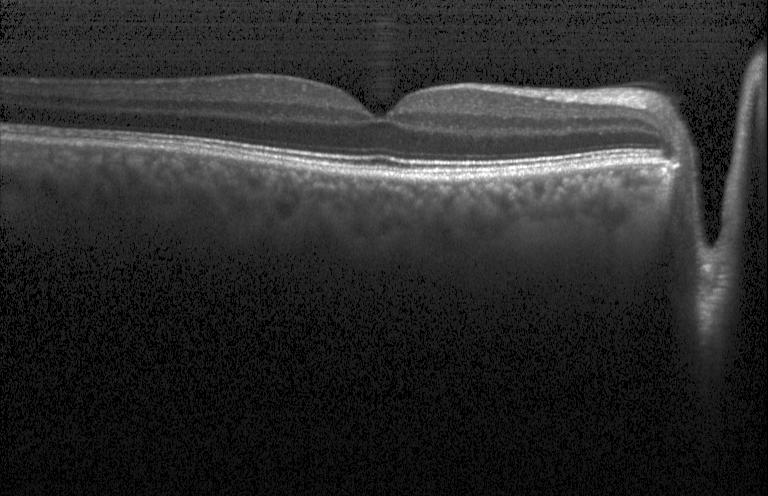

Spectral-domain OCT B-scan: no CNV, no DME, and no drusen.